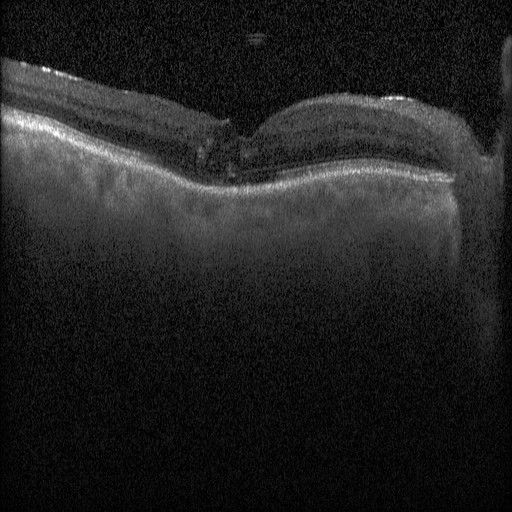

Optical coherence tomography B-scan; fovea-centered
Macular OCT: diabetic macular edema (DME).